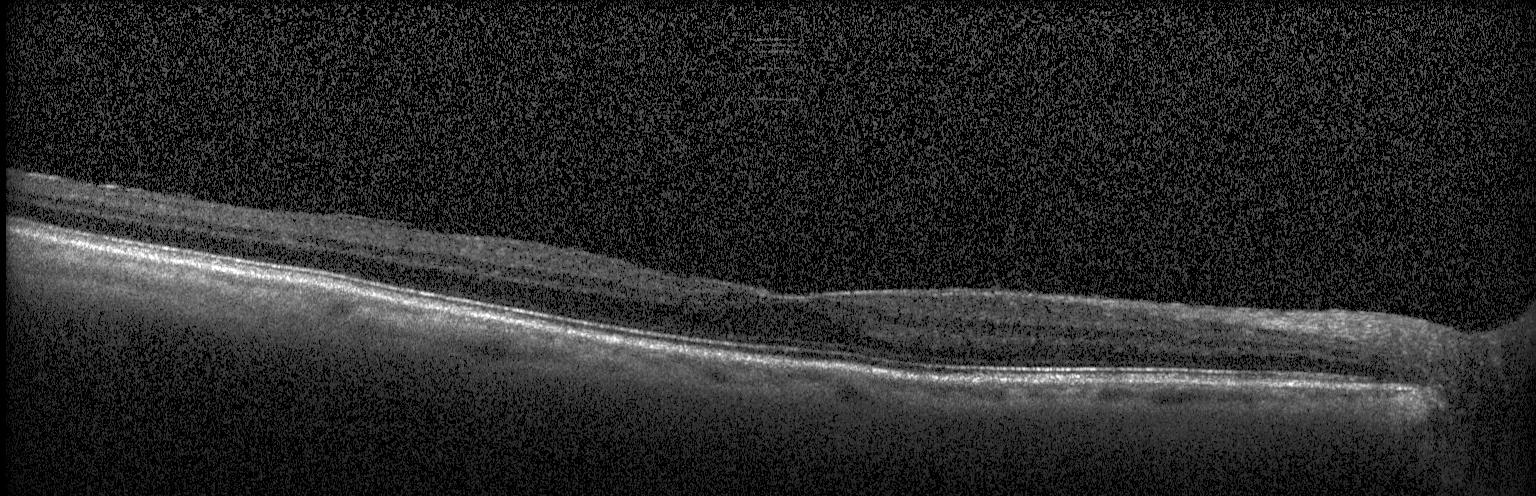

OCT B-scan · acquired on a Heidelberg Spectralis · SD-OCT · horizontal scan through the fovea. OCT finding: no choroidal neovascularization, no diabetic macular edema, and no drusen.